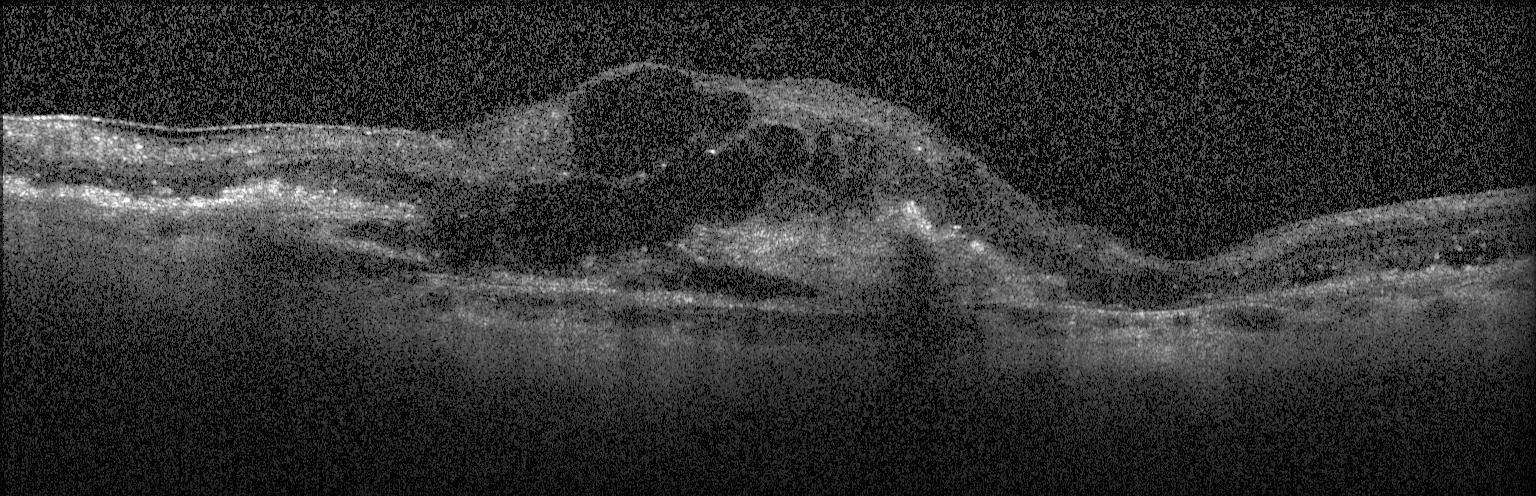 Centered on the fovea; spectral-domain OCT; Heidelberg Spectralis; optical coherence tomography scan — Dx: choroidal neovascularization.